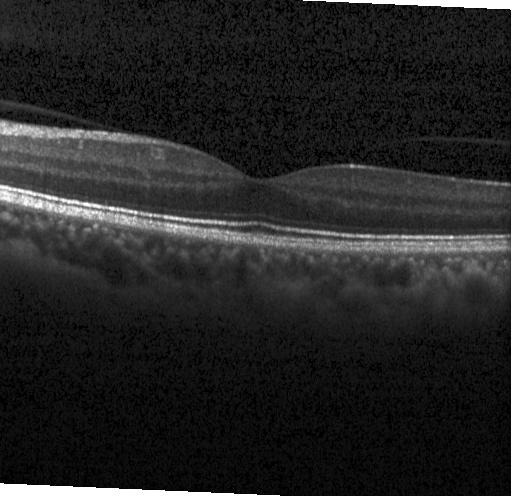
Through the macula, retinal OCT B-scan — Impression: no CNV, DME, or drusen.